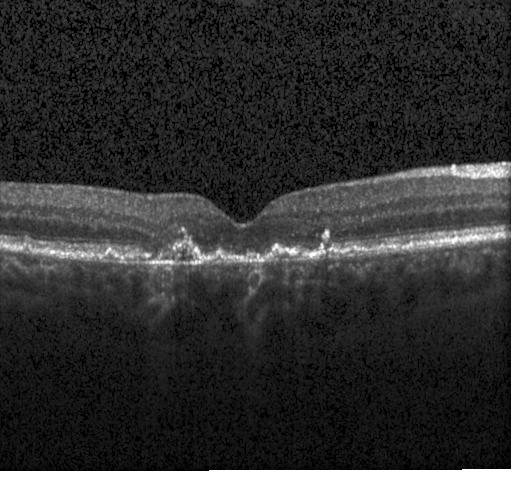 Impression: CNV.